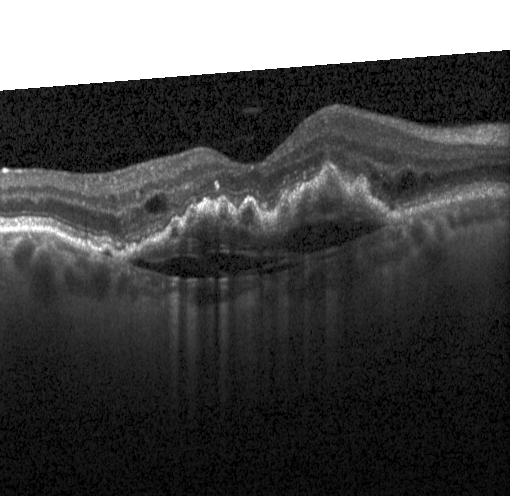 Macular OCT demonstrating a choroidal neovascular membrane.